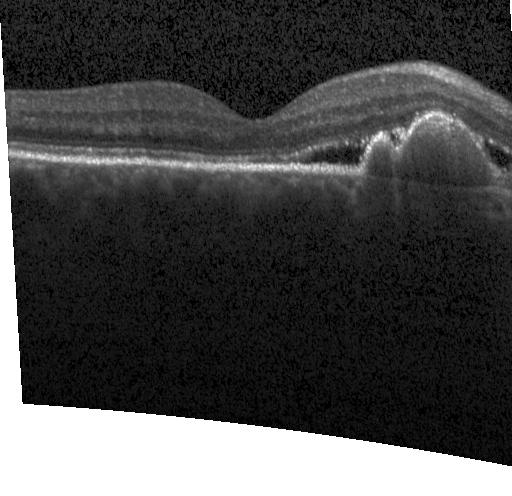 OCT B-scan — OCT finding: choroidal neovascularization.